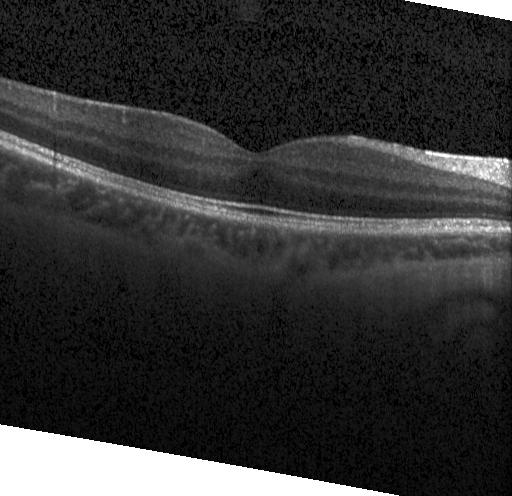 Centered on the fovea, acquired on a Heidelberg Spectralis, spectral-domain optical coherence tomography, OCT B-scan
This B-scan demonstrates no choroidal neovascularization, diabetic macular edema, or drusen.